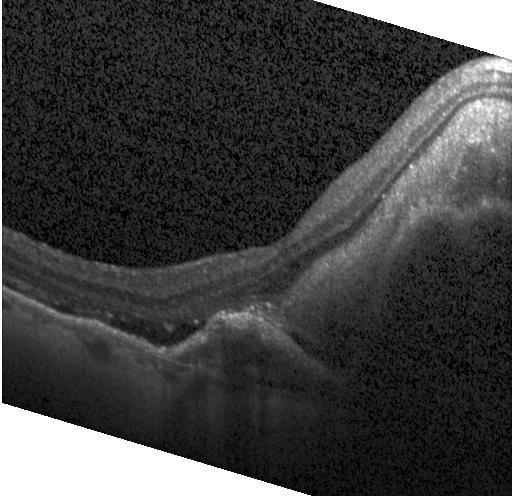 OCT line scan. Assessment: a choroidal neovascular membrane.